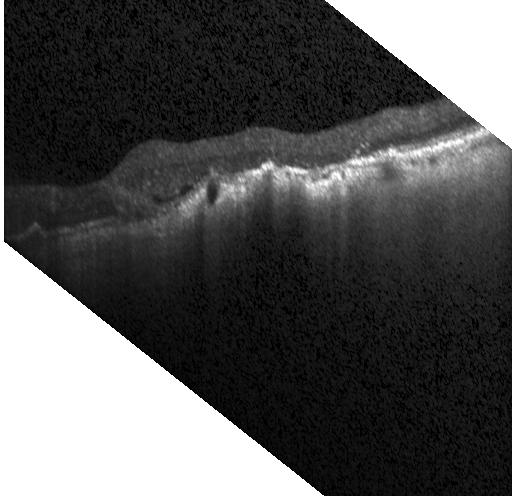 OCT line scan — Macular OCT: a choroidal neovascular membrane.